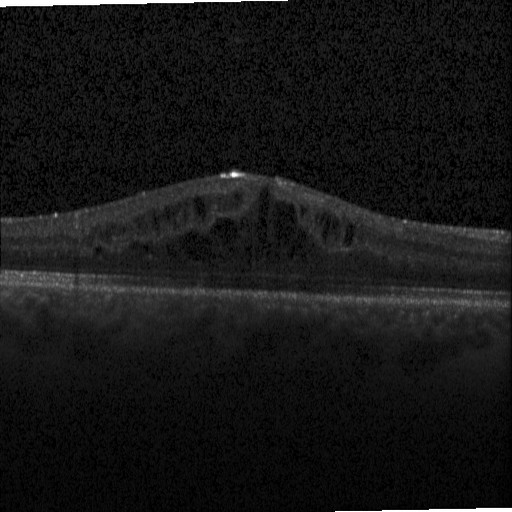

Optical coherence tomography B-scan. OCT finding: diabetic macular edema (DME).